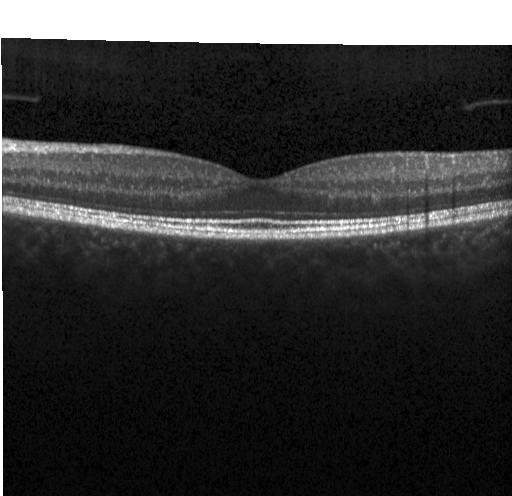
No CNV, DME, or drusen.